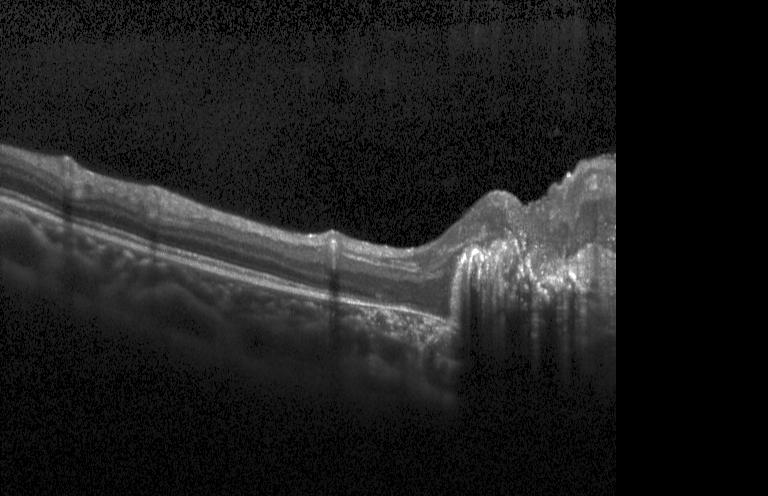

Spectral-domain optical coherence tomography, retinal OCT B-scan, fovea-centered, Heidelberg Spectralis OCT system. Finding: a choroidal neovascular membrane.